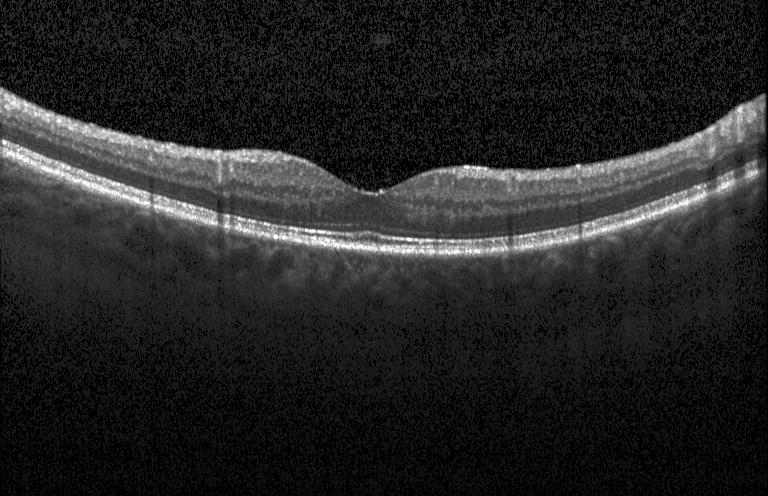
Heidelberg Spectralis · OCT line scan · fovea-centered · SD-OCT — Dx: no evidence of CNV, DME, or drusen.